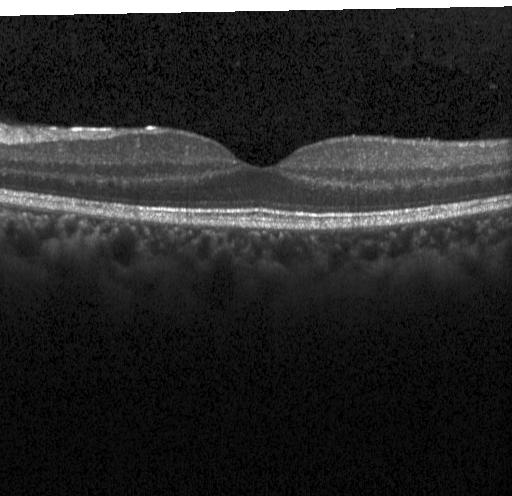

Retinal OCT cross-section · instrument: Heidelberg Spectralis · centered on the fovea · SD-OCT.
Finding: no choroidal neovascularization, no diabetic macular edema, and no drusen.